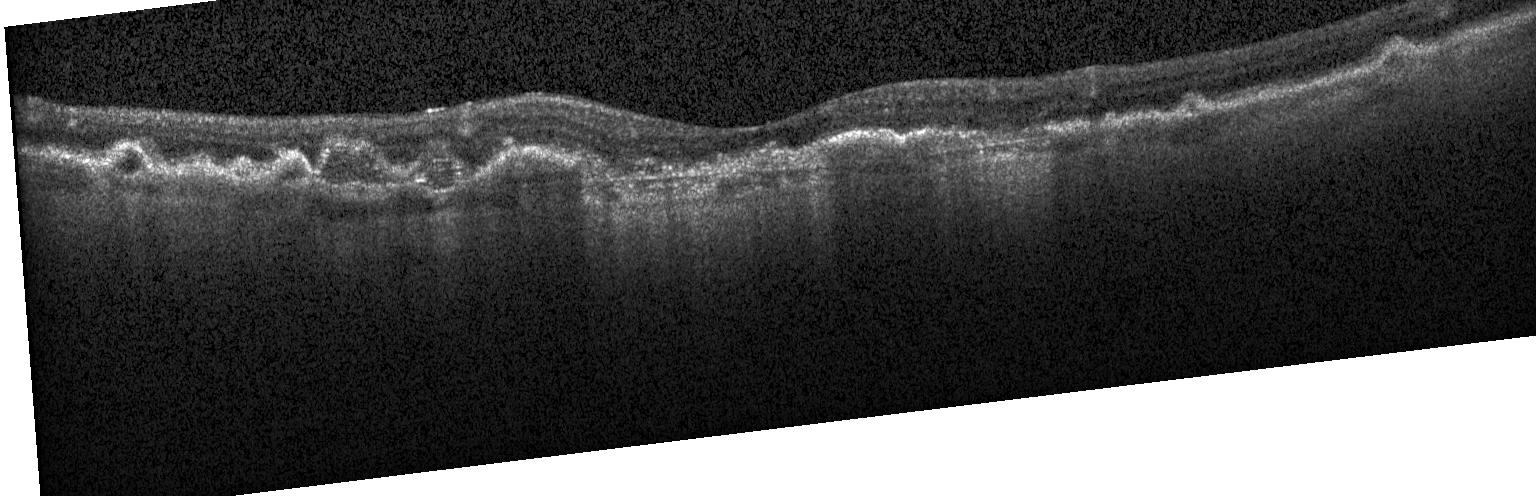

Retinal OCT B-scan; spectral-domain OCT; Heidelberg Spectralis OCT system; macular scan.
Macular OCT: a choroidal neovascular membrane.